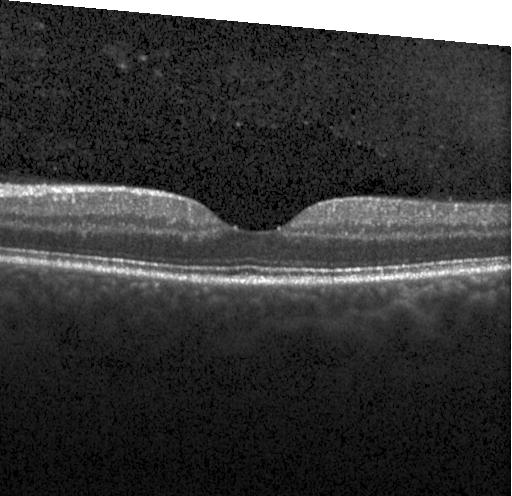 OCT B-scan. Macular scan. Spectral-domain OCT. Heidelberg Spectralis OCT system — Diagnosis: no evidence of choroidal neovascularization, diabetic macular edema, or drusen.